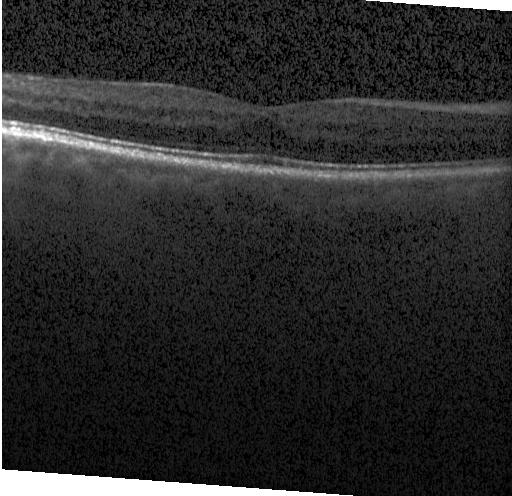 Macular OCT: no choroidal neovascularization, no diabetic macular edema, and no drusen.